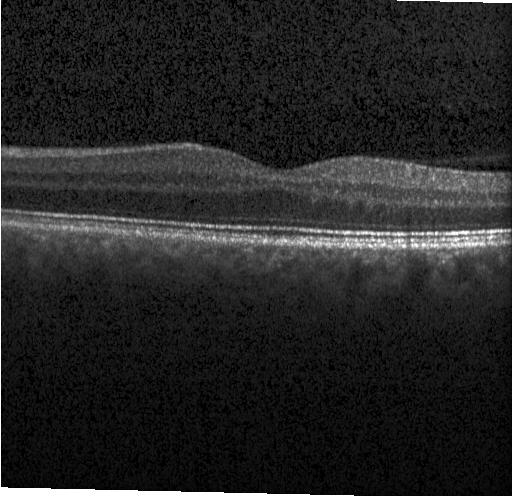

Neither choroidal neovascularization, diabetic macular edema, nor drusen.